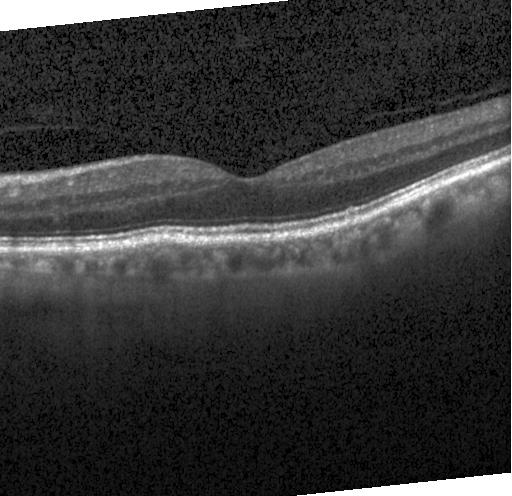
Impression: no choroidal neovascularization, no diabetic macular edema, and no drusen.